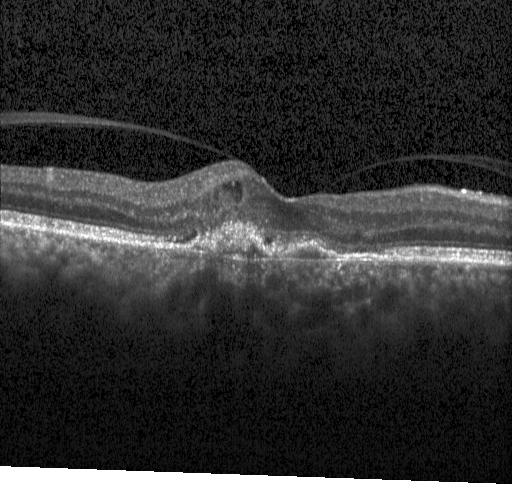 OCT B-scan
Finding: a choroidal neovascular membrane.